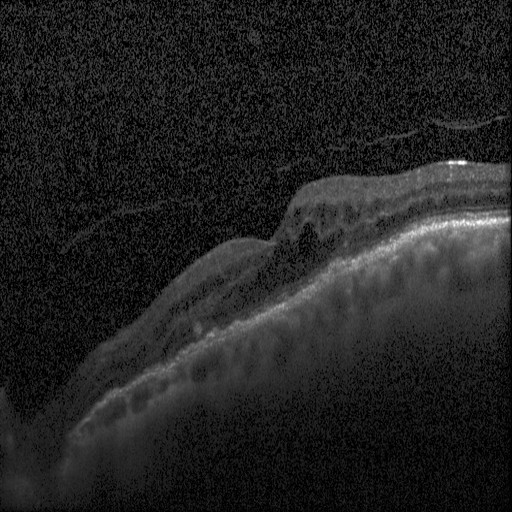 Fovea-centered; Heidelberg Spectralis; spectral-domain OCT; OCT B-scan. Finding: diabetic macular edema (DME).